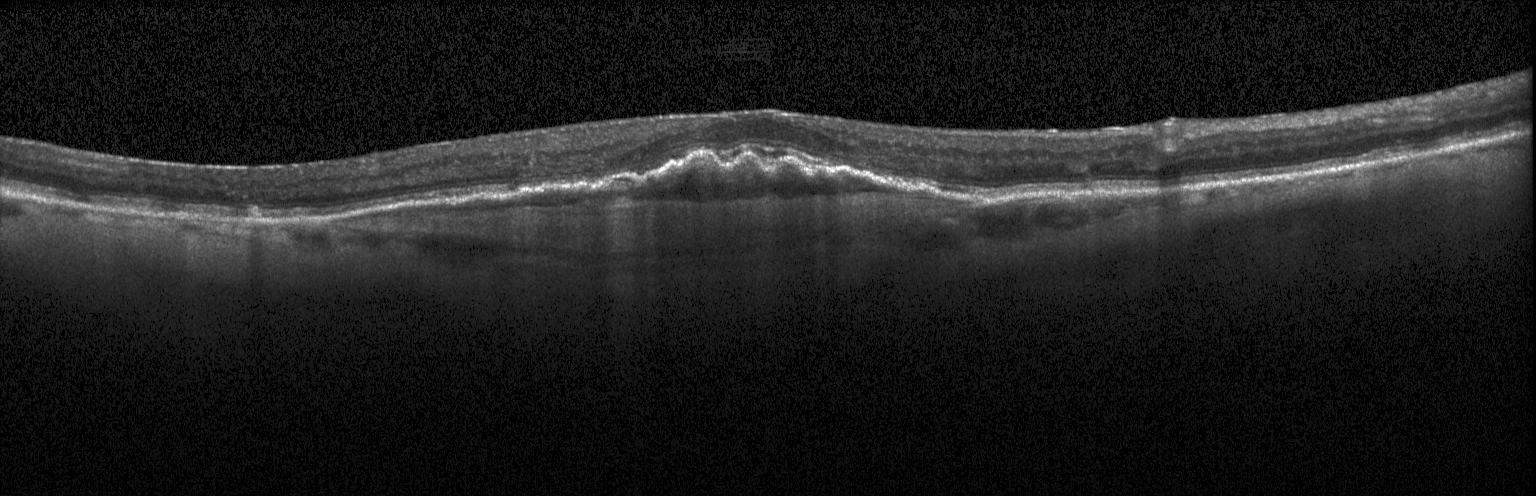

Diagnosis: choroidal neovascularization (CNV).